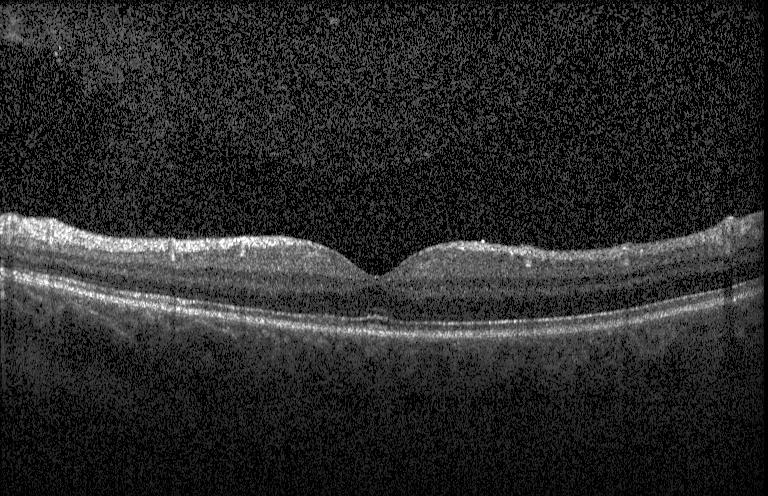

Impression: no choroidal neovascularization, diabetic macular edema, or drusen.